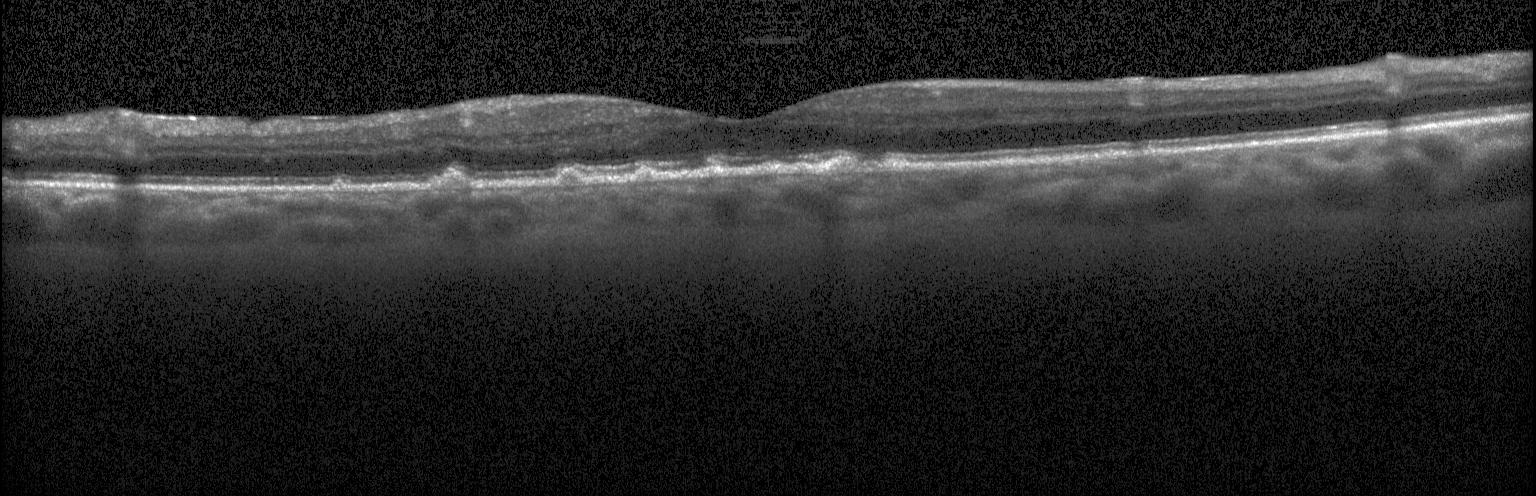
Spectral-domain optical coherence tomography · instrument: Heidelberg Spectralis · macular scan · retinal OCT cross-section — The scan shows drusen.